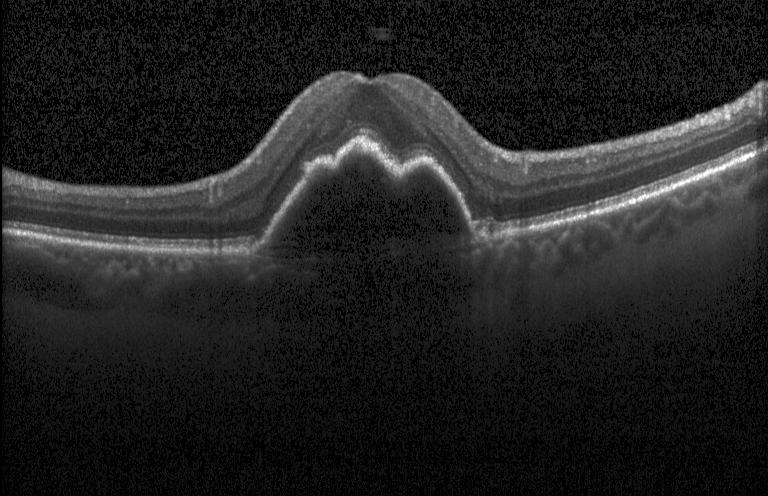

Acquired on a Heidelberg Spectralis, optical coherence tomography scan, spectral-domain OCT.
Impression: choroidal neovascularization.